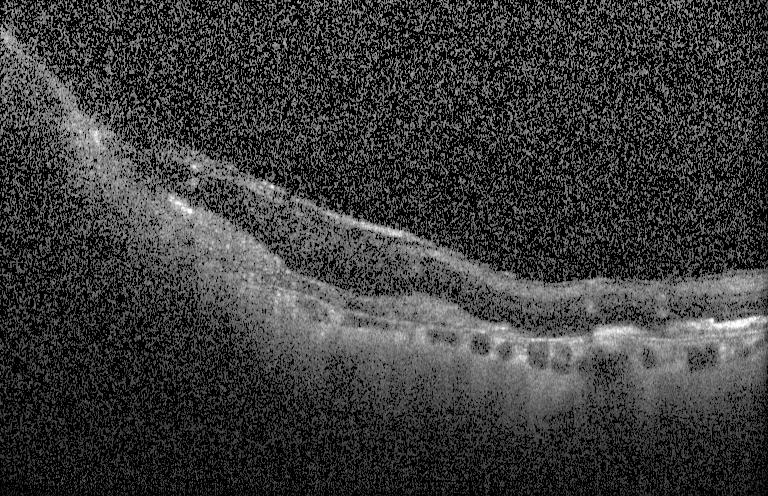
OCT scan showing a choroidal neovascular membrane.